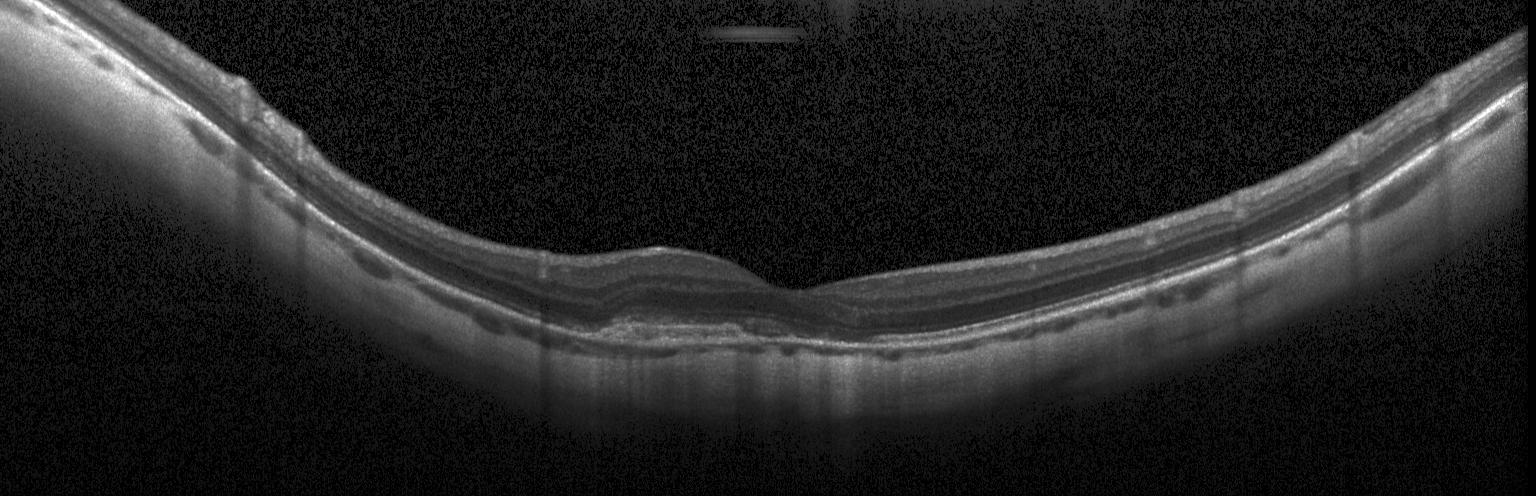
Retinal OCT cross-section, acquired on a Heidelberg Spectralis
Diagnosis: CNV.